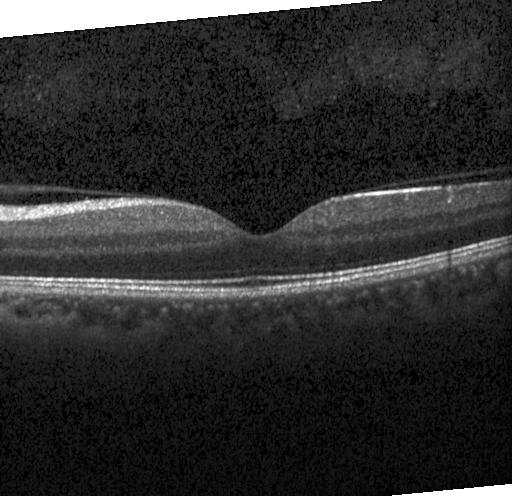 Impression: neither choroidal neovascularization, diabetic macular edema, nor drusen.